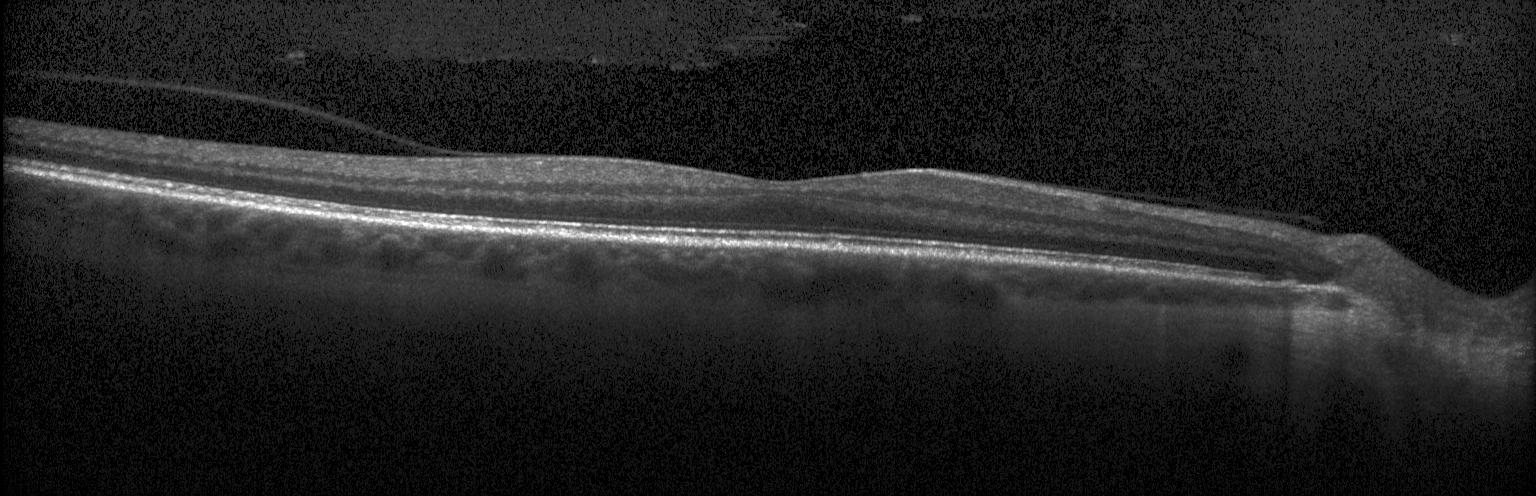

Finding: no choroidal neovascularization, diabetic macular edema, or drusen.